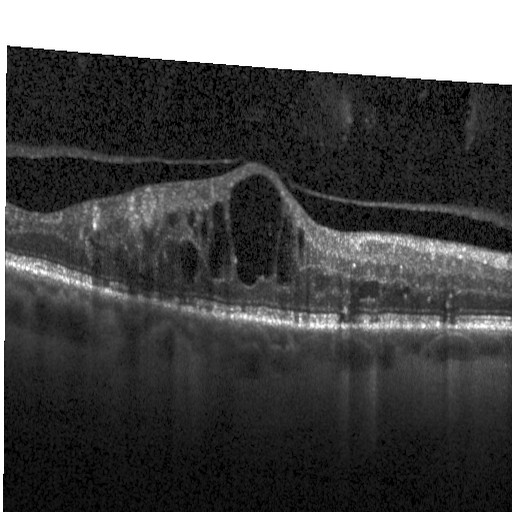

Spectral-domain optical coherence tomography; retinal OCT cross-section — Assessment: DME.